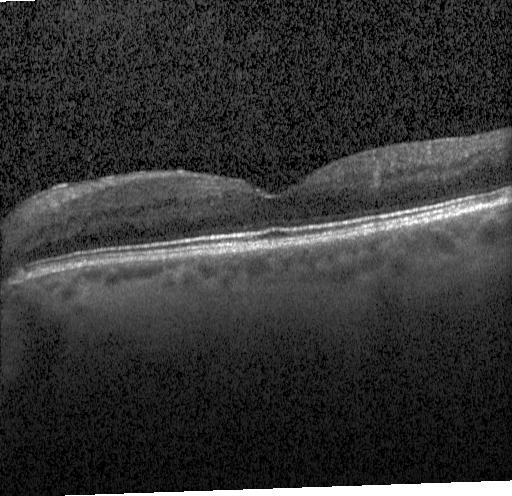

Through the macula · retinal OCT B-scan · spectral-domain OCT
Macular OCT: neither choroidal neovascularization, diabetic macular edema, nor drusen.